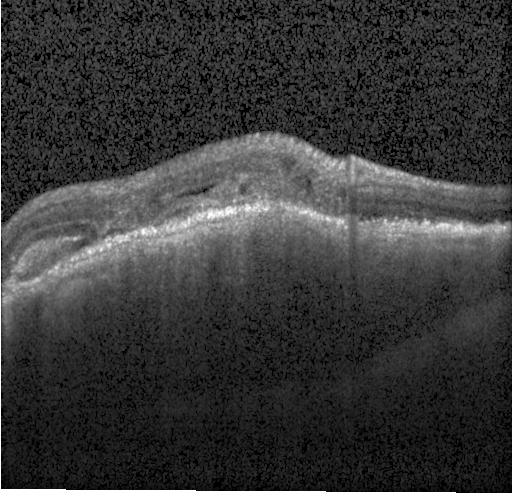
Horizontal scan through the fovea; instrument: Heidelberg Spectralis; spectral-domain optical coherence tomography; OCT B-scan. Diagnosis: a choroidal neovascular membrane.